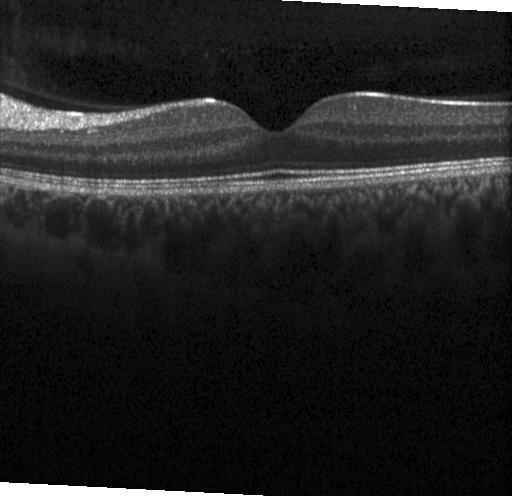
Macular OCT demonstrating no evidence of choroidal neovascularization, diabetic macular edema, or drusen.